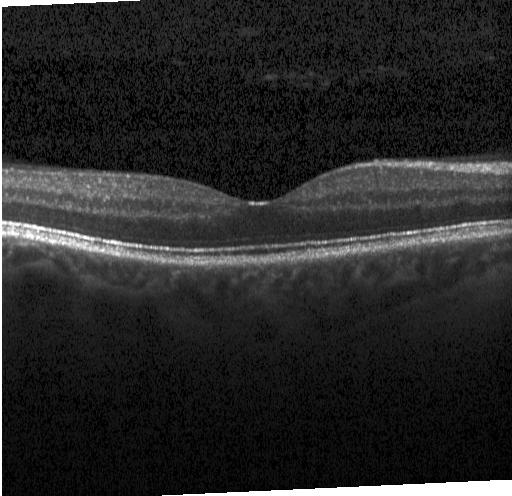 Finding: neither choroidal neovascularization, diabetic macular edema, nor drusen.